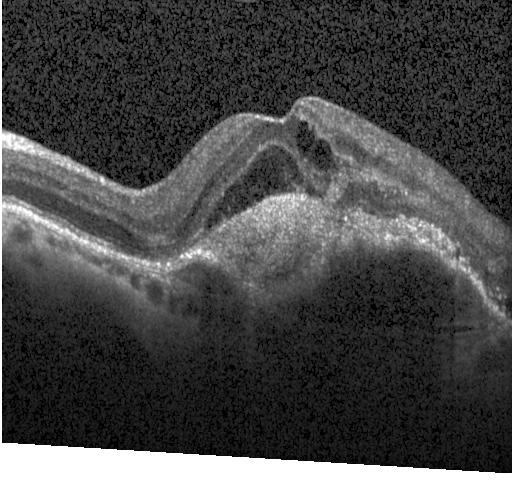
Impression: CNV.